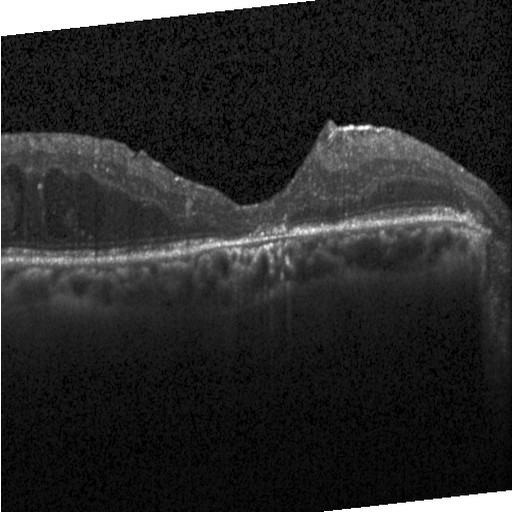

Retinal OCT cross-section, instrument: Heidelberg Spectralis, through the macula
Dx: DME.